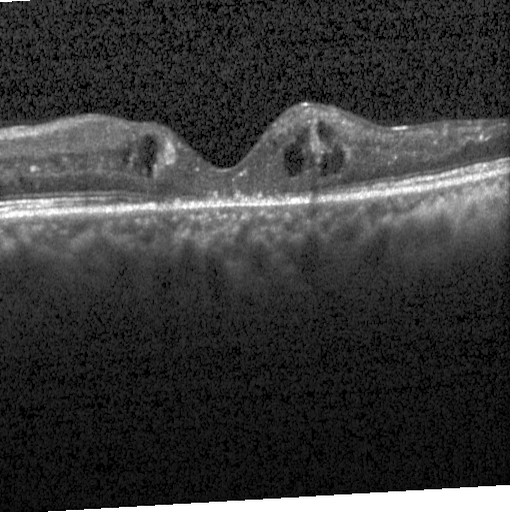

SD-OCT · Heidelberg Spectralis OCT system · optical coherence tomography B-scan · macular scan.
Impression: diabetic macular edema.